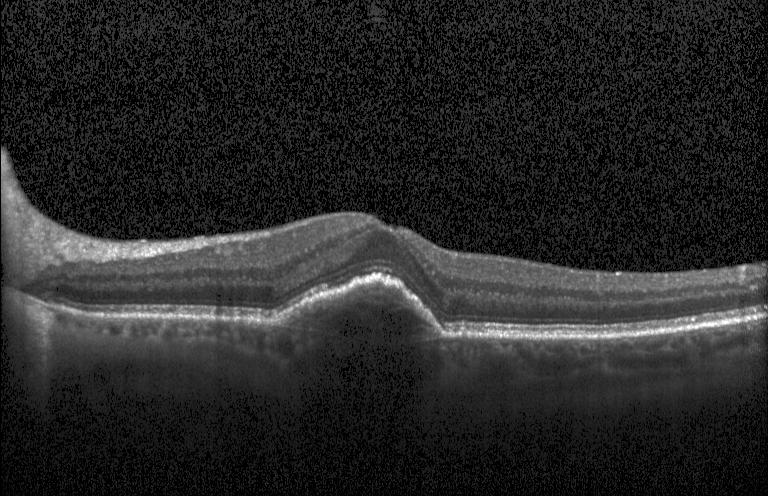 Retinal OCT cross-section · SD-OCT. Diagnosis: CNV.